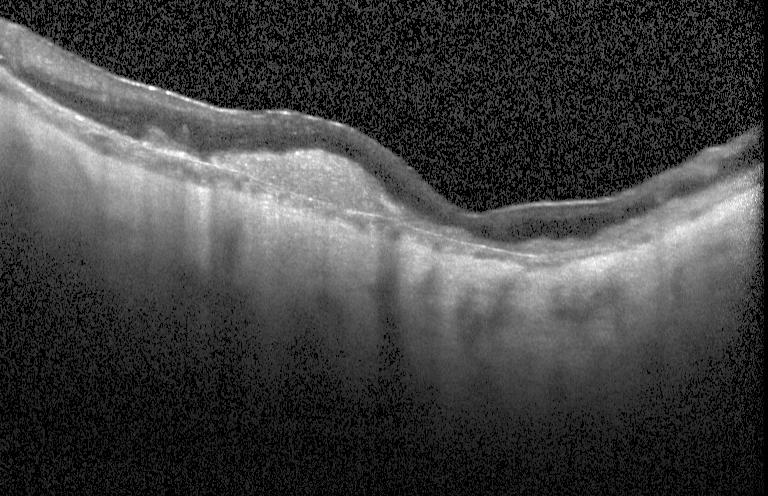
Optical coherence tomography B-scan. Horizontal scan through the fovea. Finding: a choroidal neovascular membrane.